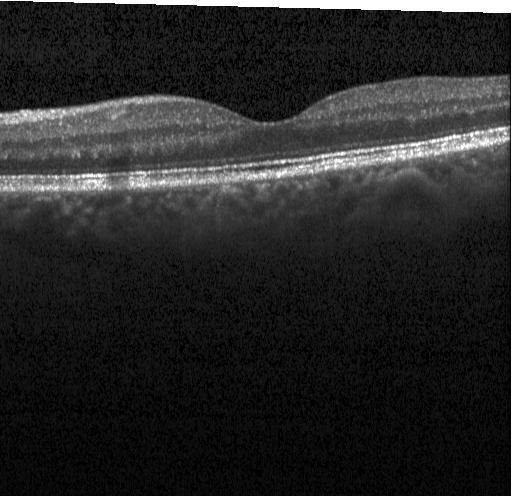 Retinal OCT B-scan.
Diagnosis: no choroidal neovascularization, no diabetic macular edema, and no drusen.